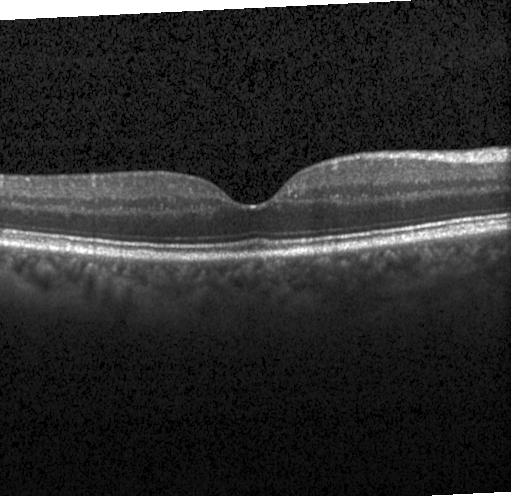
OCT line scan. Spectral-domain OCT. Fovea-centered. Finding: neither CNV, DME, nor drusen.